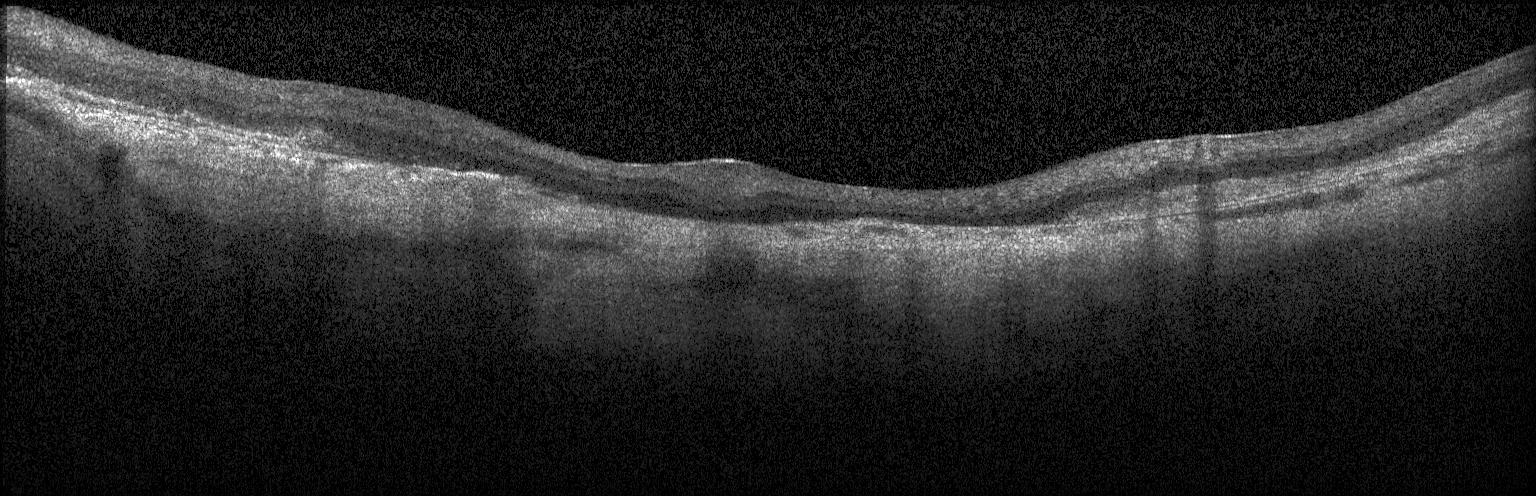

Spectral-domain OCT B-scan: a choroidal neovascular membrane.